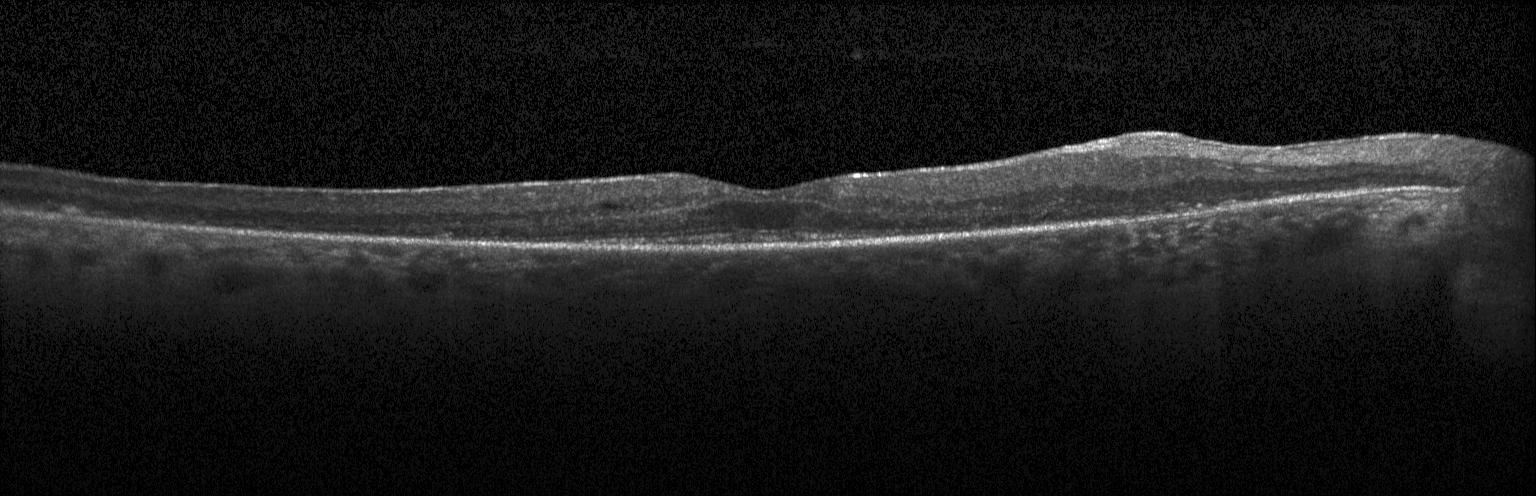 SD-OCT · OCT B-scan · Heidelberg Spectralis — Finding: diabetic macular edema.